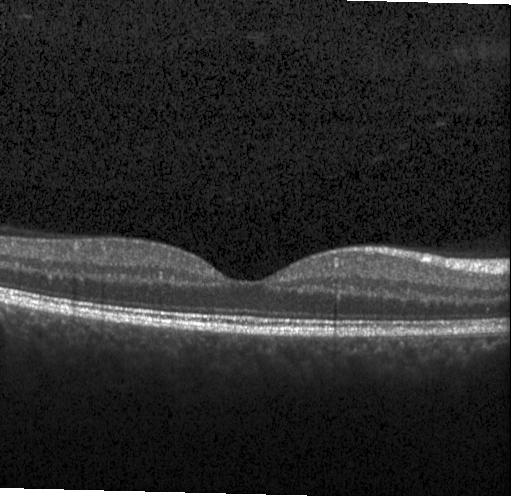

Retinal OCT cross-section showing no evidence of CNV, DME, or drusen.